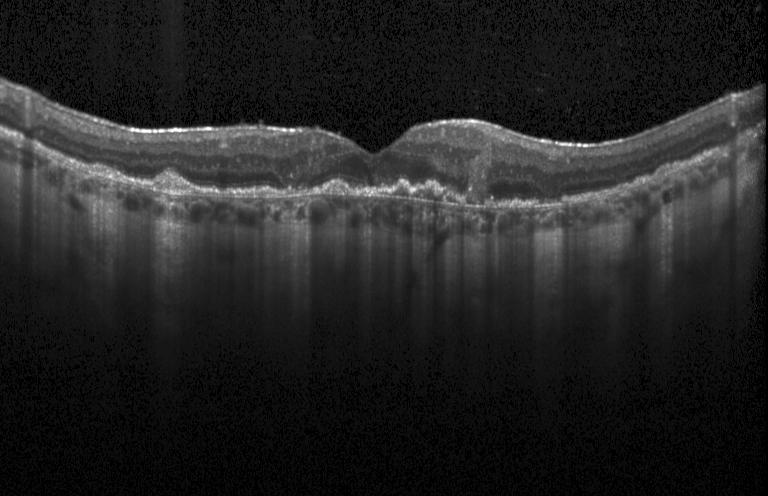 OCT B-scan showing CNV.